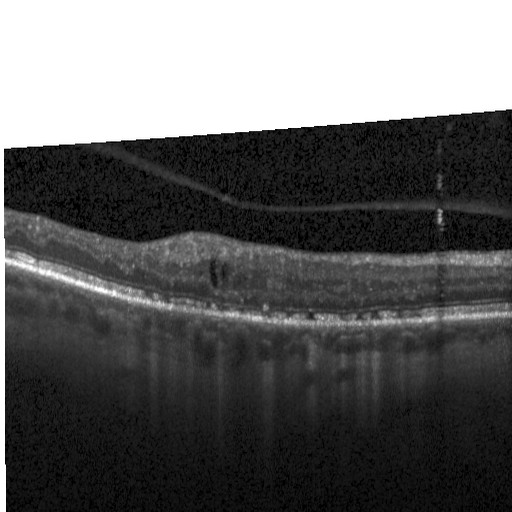

Heidelberg Spectralis. OCT line scan. Through the macula
DME.